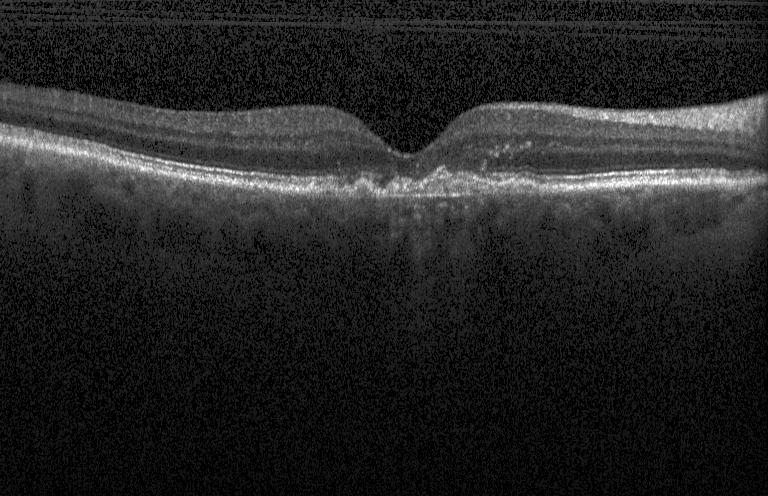 OCT B-scan · fovea-centered · spectral-domain optical coherence tomography. Dx: a choroidal neovascular membrane.